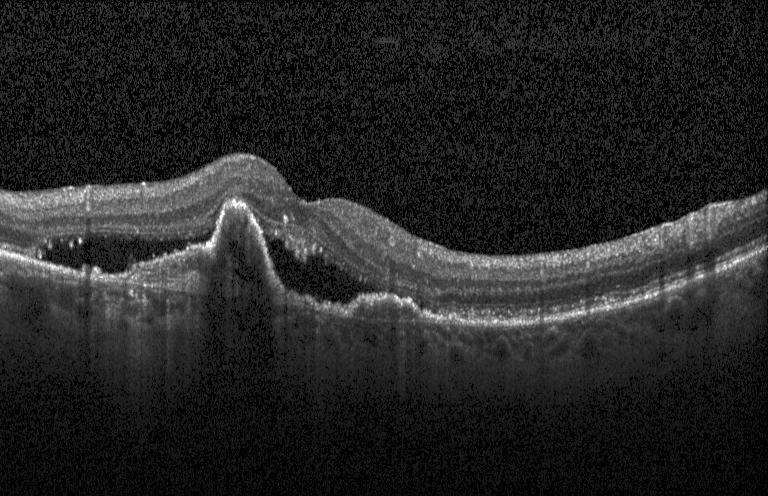

OCT B-scan showing a choroidal neovascular membrane.